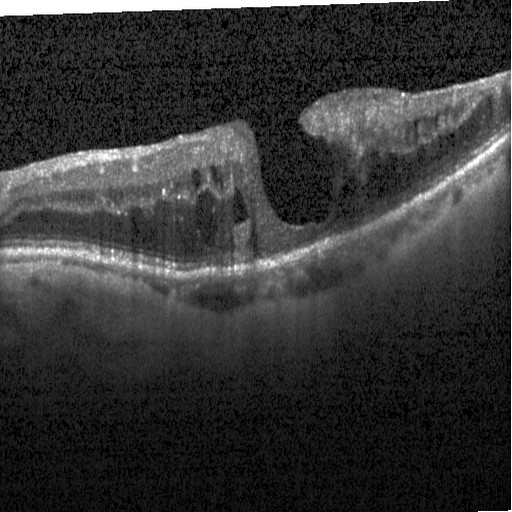
Optical coherence tomography B-scan
OCT finding: DME.